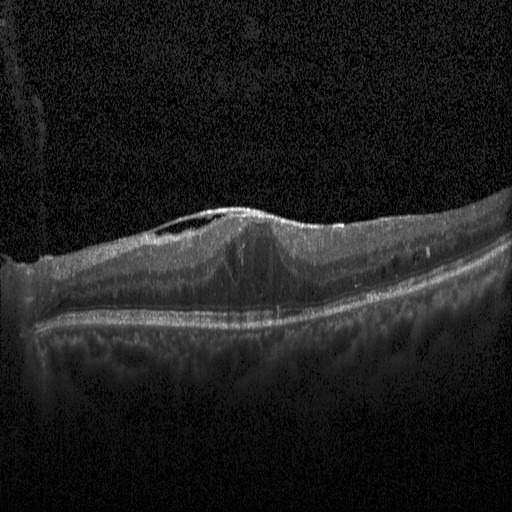 OCT B-scan showing diabetic macular edema.